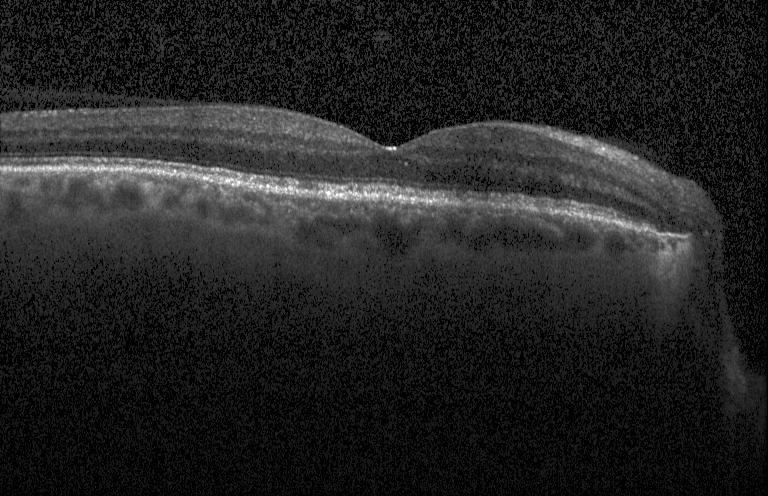

Finding: no evidence of choroidal neovascularization, diabetic macular edema, or drusen.